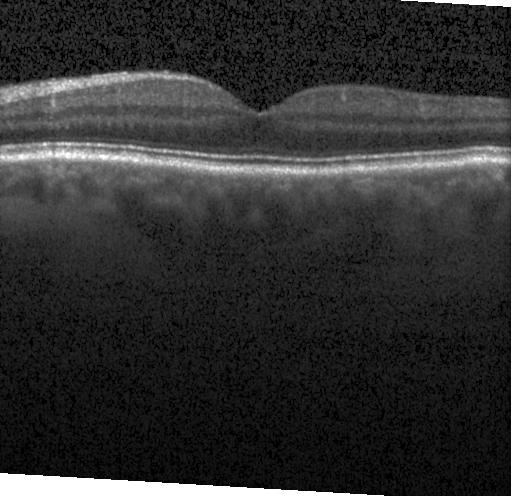
Optical coherence tomography B-scan — Finding: no choroidal neovascularization, diabetic macular edema, or drusen.